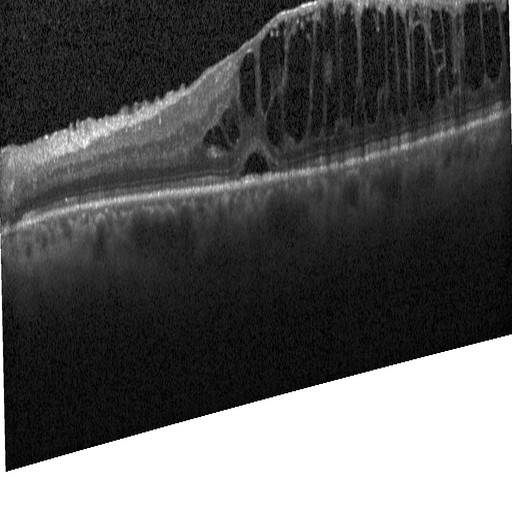

OCT line scan; horizontal scan through the fovea. The scan shows diabetic macular edema (DME).